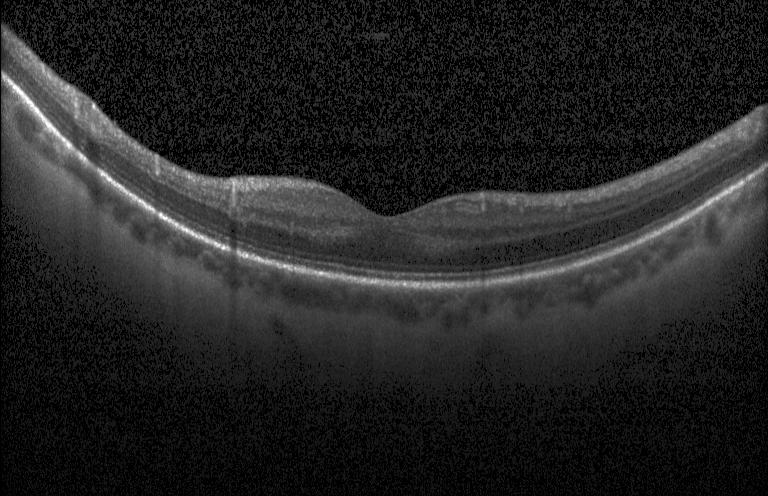

Macular OCT: neither choroidal neovascularization, diabetic macular edema, nor drusen.